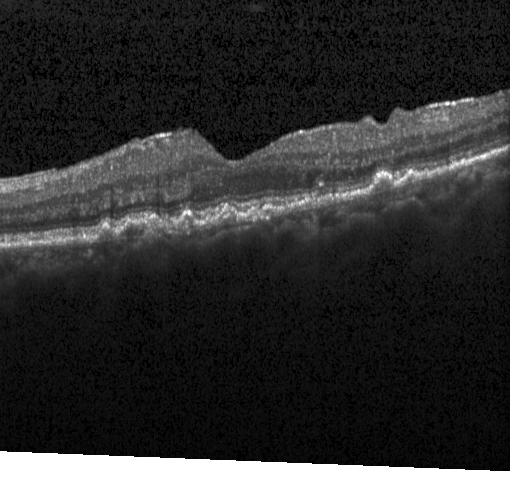

Centered on the fovea. Retinal OCT cross-section.
Impression: sub-RPE drusenoid deposits.